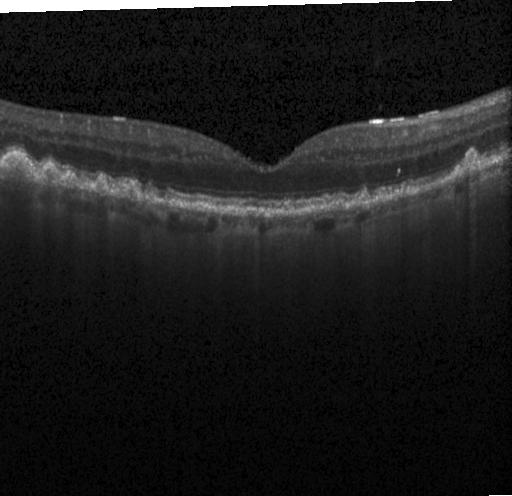 Spectral-domain OCT B-scan: drusen.